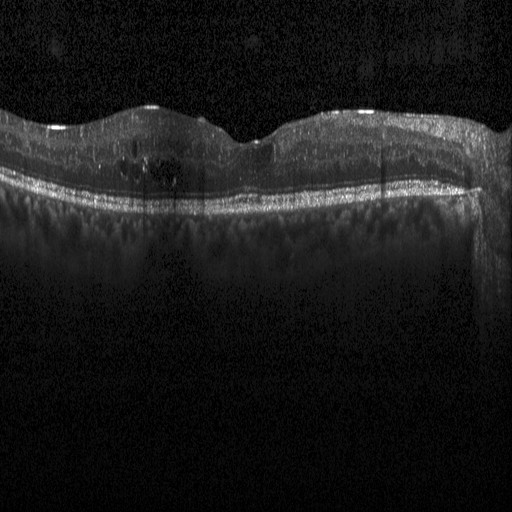

The scan shows DME.